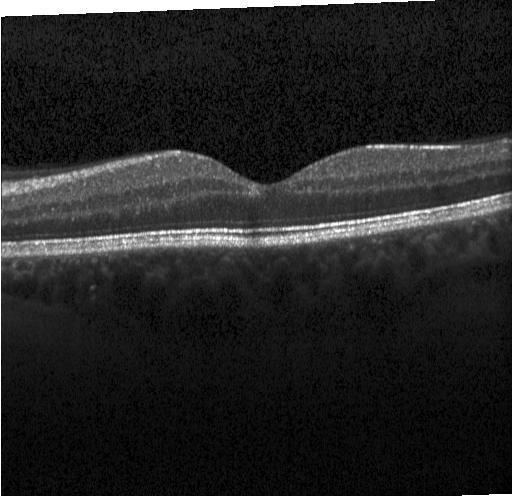 Impression: no choroidal neovascularization, diabetic macular edema, or drusen.